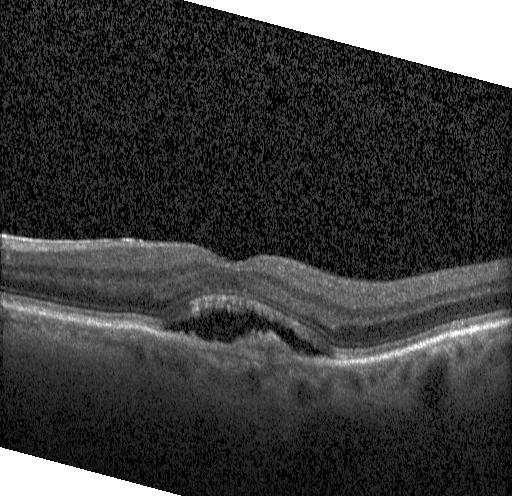
Macular OCT demonstrating a choroidal neovascular membrane.